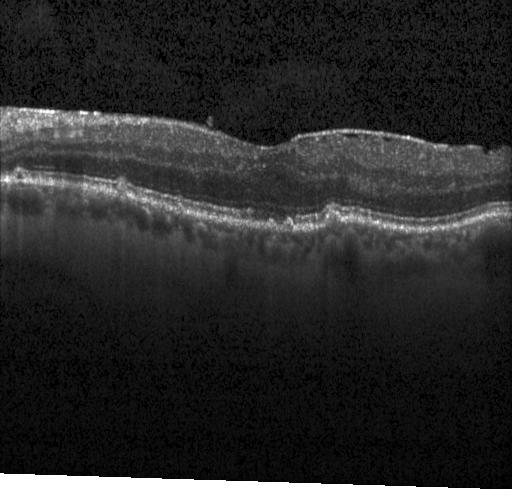
Macular scan; OCT B-scan; spectral-domain optical coherence tomography; Heidelberg Spectralis
Impression: sub-RPE drusenoid deposits.